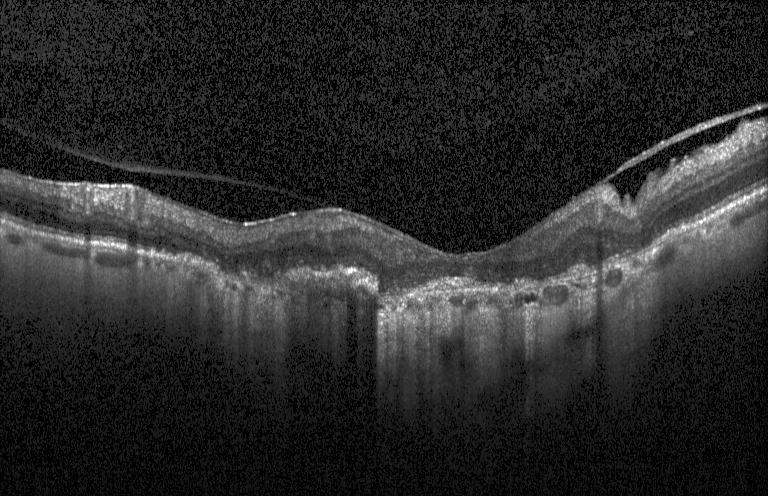 OCT B-scan showing a choroidal neovascular membrane.